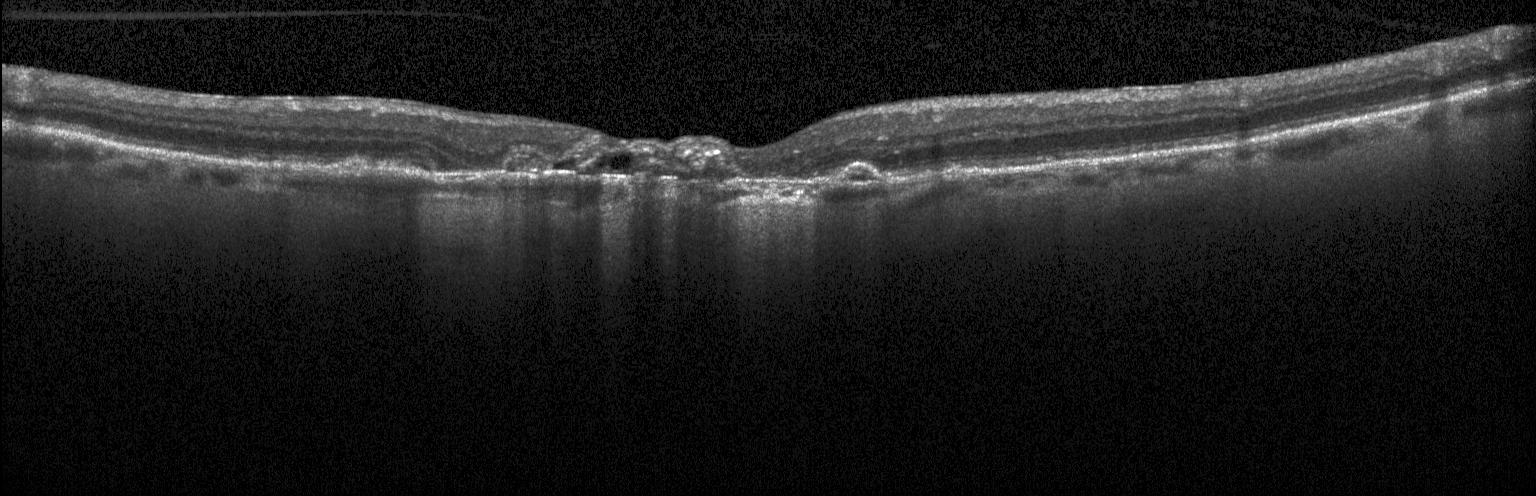 Diagnosis: choroidal neovascularization (CNV).